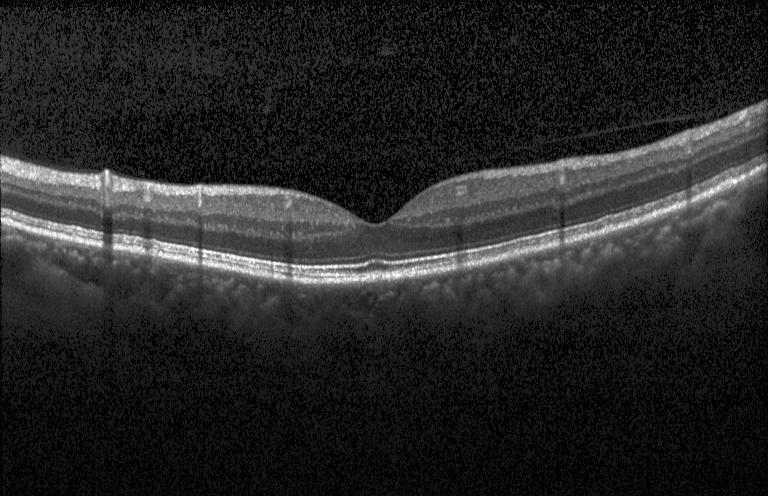
Centered on the fovea · SD-OCT · OCT line scan
This B-scan demonstrates no CNV, DME, or drusen.